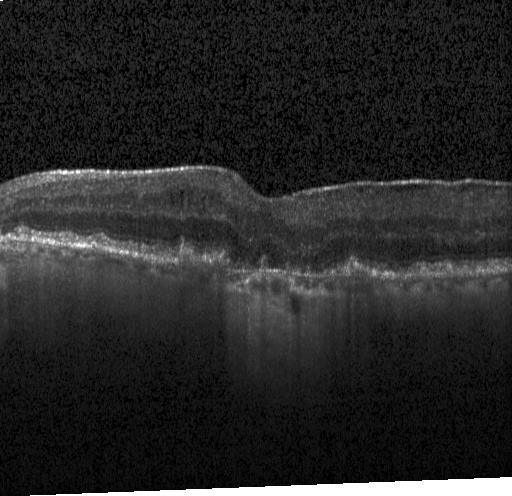 Retinal OCT cross-section
Diagnosis: a choroidal neovascular membrane.